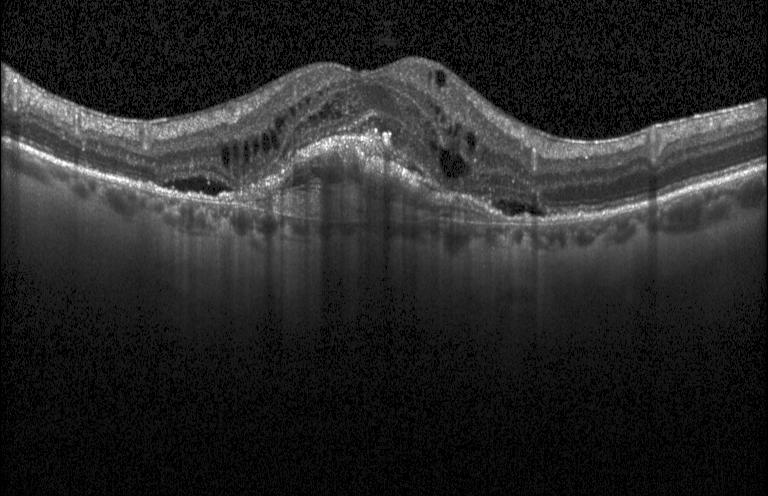

This B-scan demonstrates choroidal neovascularization.